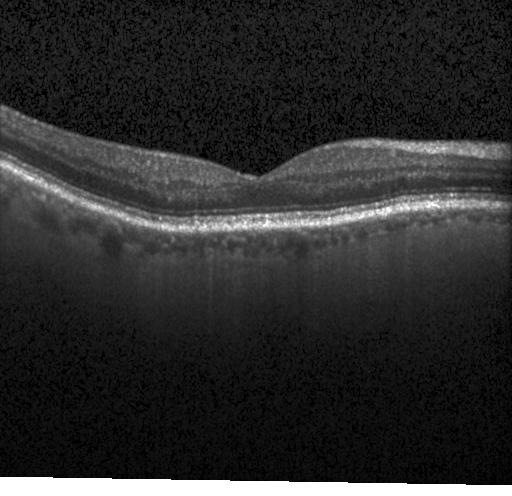 Retinal OCT B-scan
Assessment: neither CNV, DME, nor drusen.